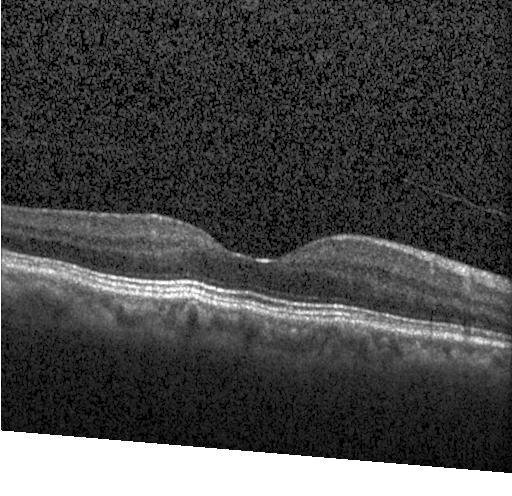
Instrument: Heidelberg Spectralis; retinal OCT B-scan; SD-OCT
OCT finding: no CNV, DME, or drusen.